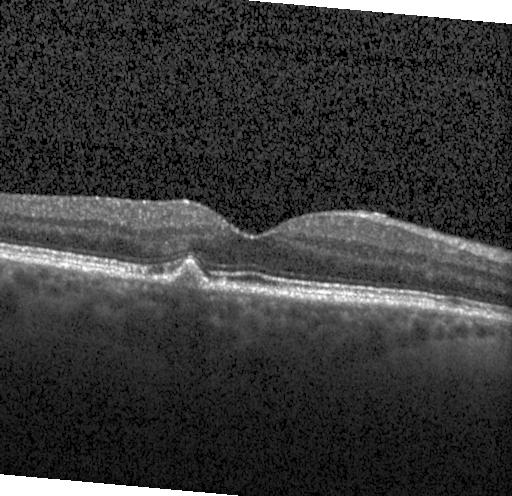
Diagnosis: drusen.